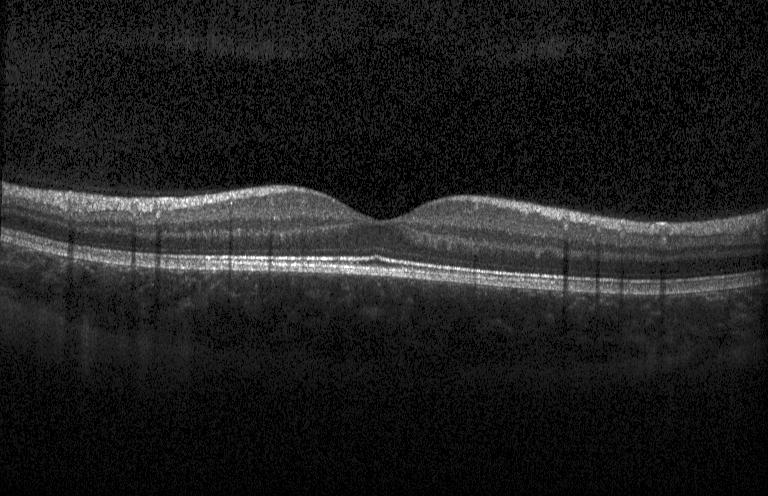 Diagnosis: no evidence of choroidal neovascularization, diabetic macular edema, or drusen.